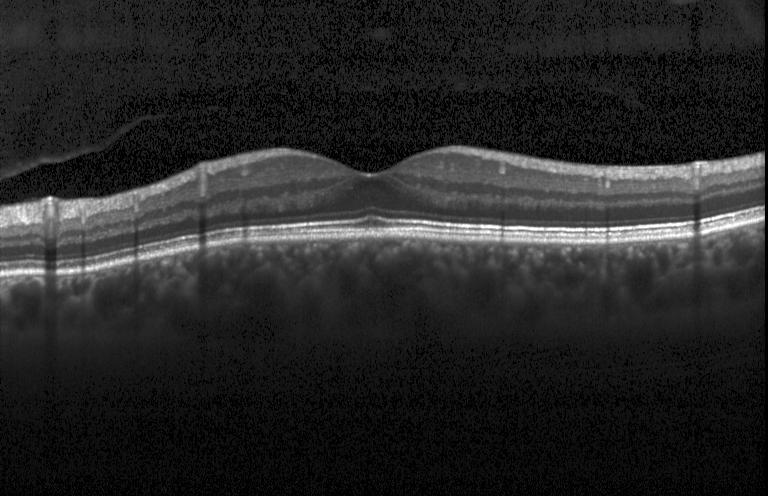

Finding: no choroidal neovascularization, no diabetic macular edema, and no drusen.